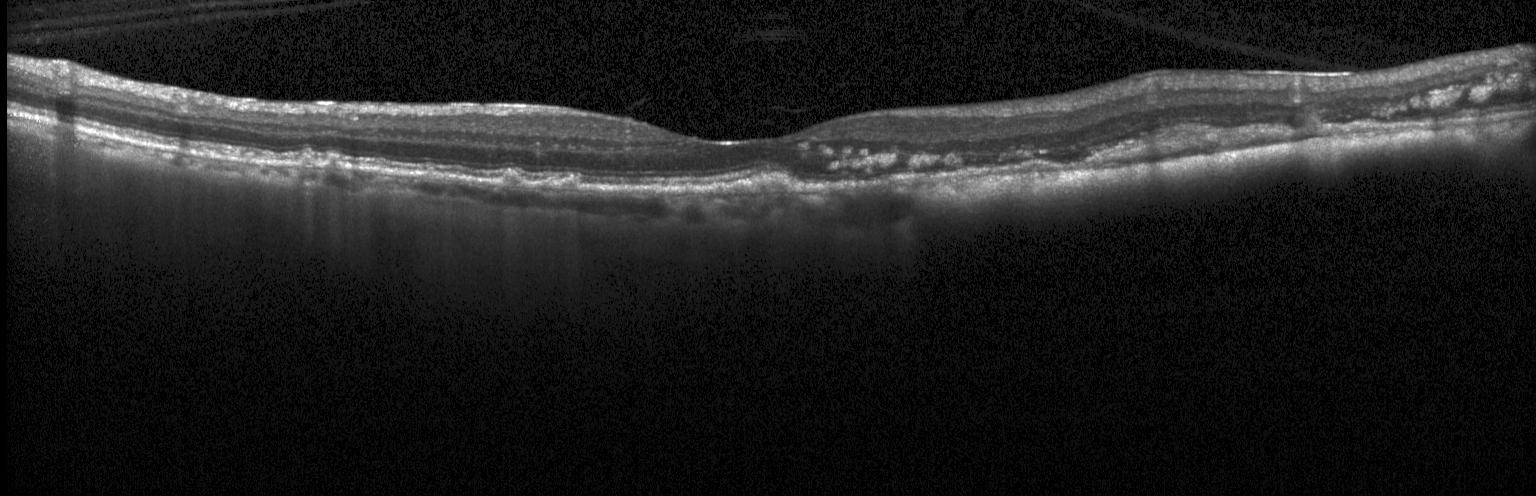 Optical coherence tomography scan.
The scan shows a choroidal neovascular membrane.